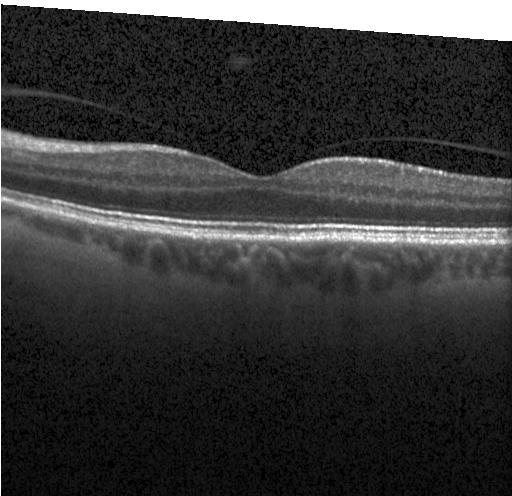 OCT B-scan showing no CNV, no DME, and no drusen.